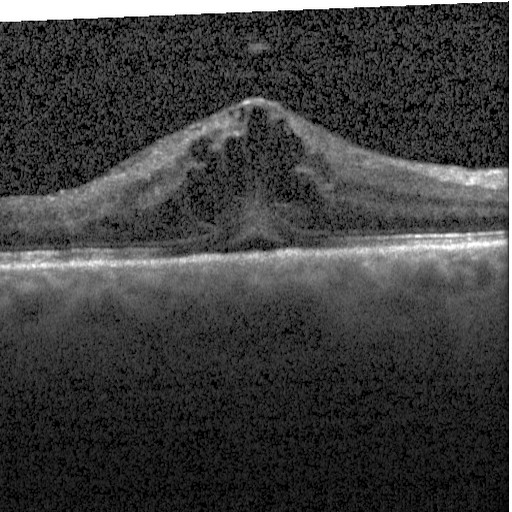 Spectral-domain OCT. Heidelberg Spectralis OCT system. Retinal OCT cross-section — Impression: diabetic macular edema (DME).